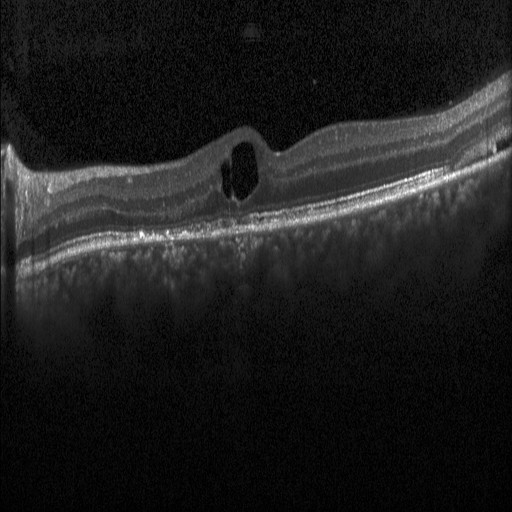 Spectral-domain optical coherence tomography; OCT B-scan; instrument: Heidelberg Spectralis.
The scan shows DME.